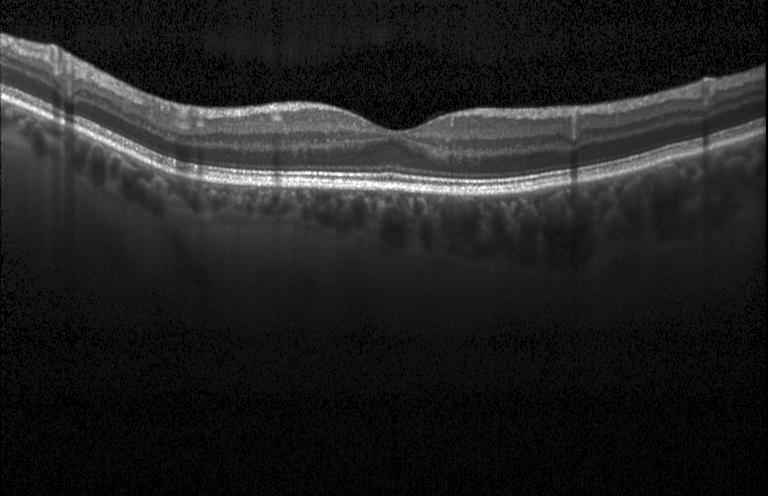 Heidelberg Spectralis OCT system · centered on the fovea · optical coherence tomography B-scan — Dx: neither CNV, DME, nor drusen.